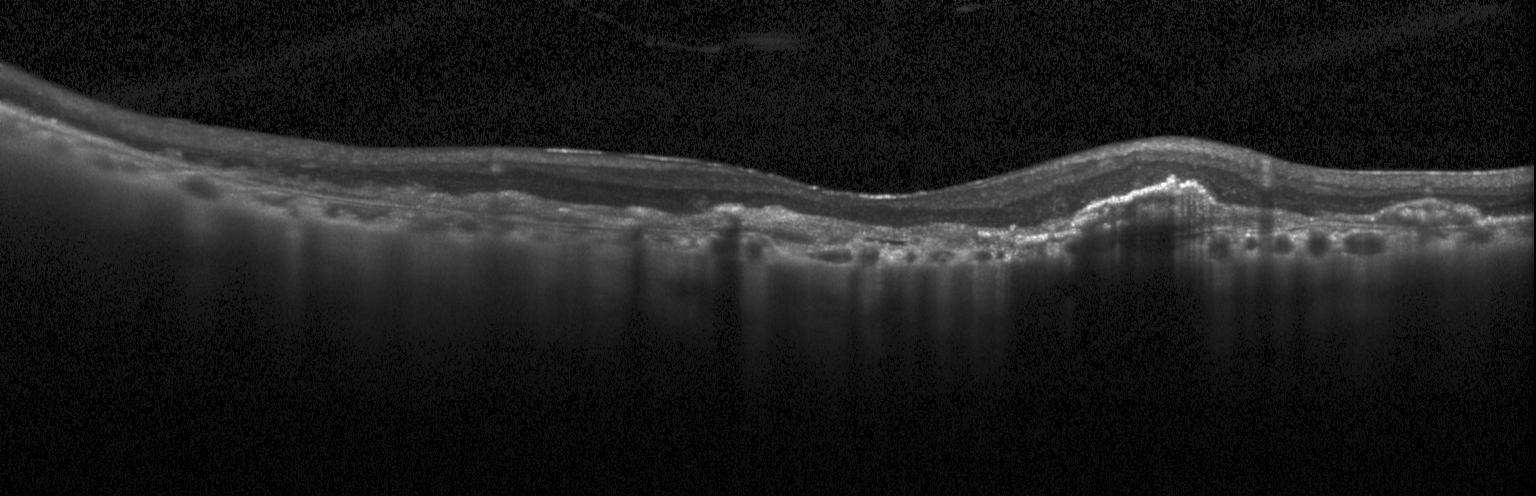
Through the macula; retinal OCT B-scan.
OCT finding: a choroidal neovascular membrane.